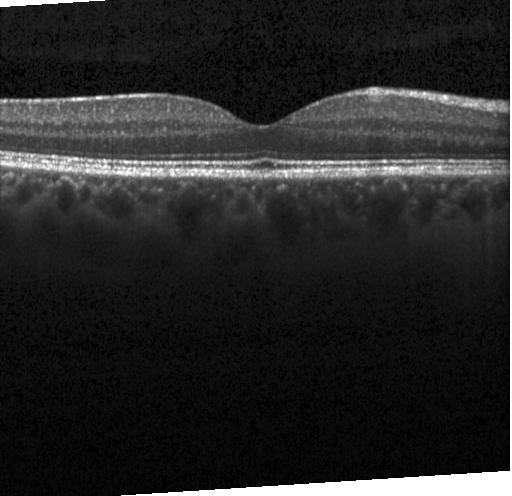
Spectral-domain OCT. Retinal OCT B-scan
Impression: no evidence of choroidal neovascularization, diabetic macular edema, or drusen.